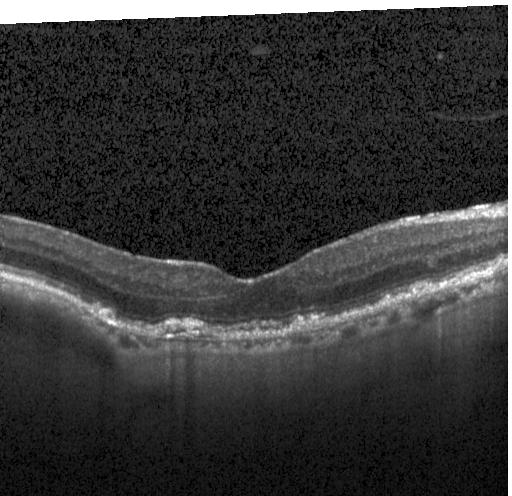
OCT scan showing choroidal neovascularization (CNV).